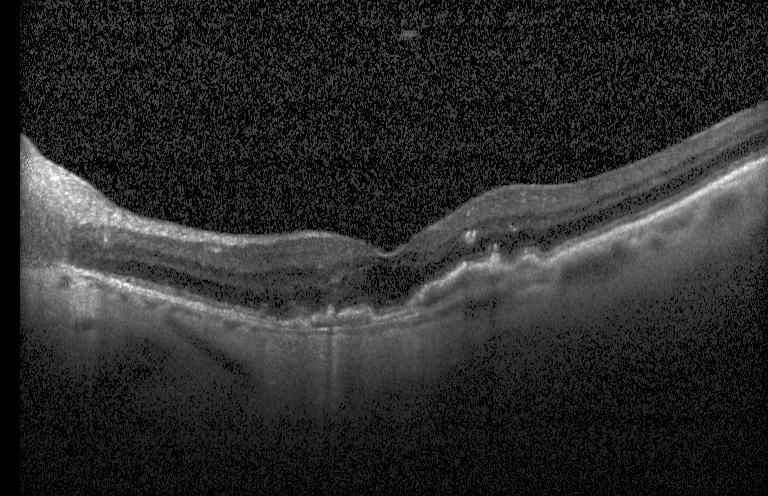 Finding: CNV.